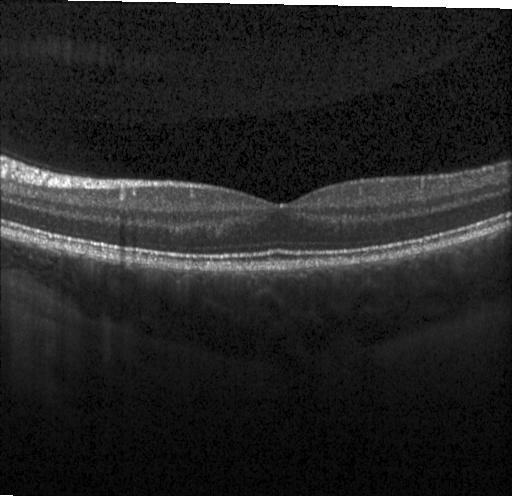
OCT scan showing no choroidal neovascularization, no diabetic macular edema, and no drusen.